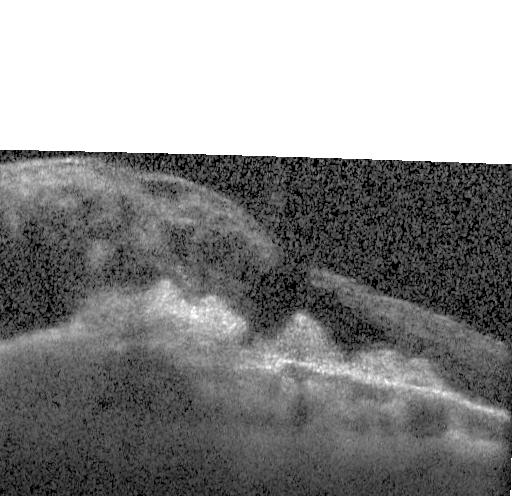
OCT B-scan; spectral-domain optical coherence tomography; Heidelberg Spectralis OCT system; macular scan — Diagnosis: CNV.